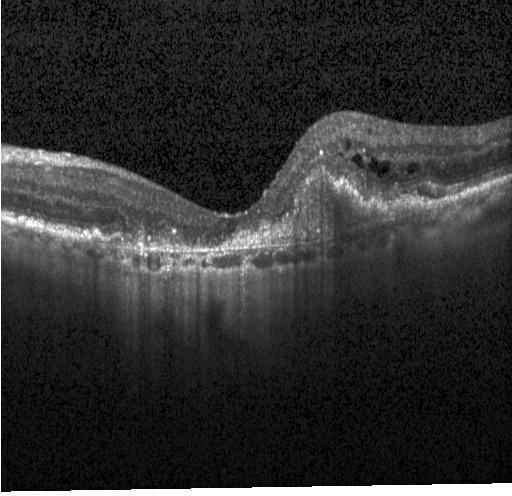 Fovea-centered · optical coherence tomography B-scan · spectral-domain OCT · instrument: Heidelberg Spectralis. Assessment: a choroidal neovascular membrane.